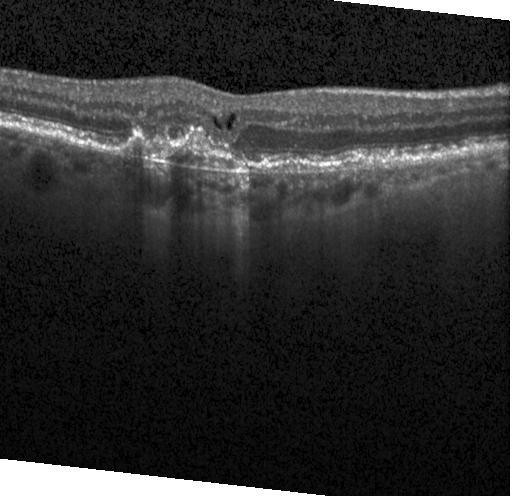
Spectral-domain OCT B-scan: choroidal neovascularization.